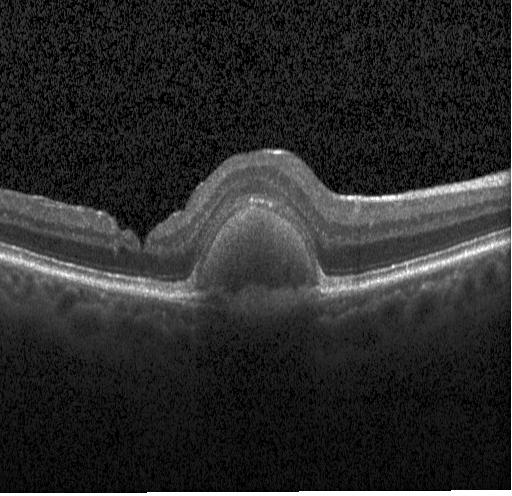
Impression: a choroidal neovascular membrane.